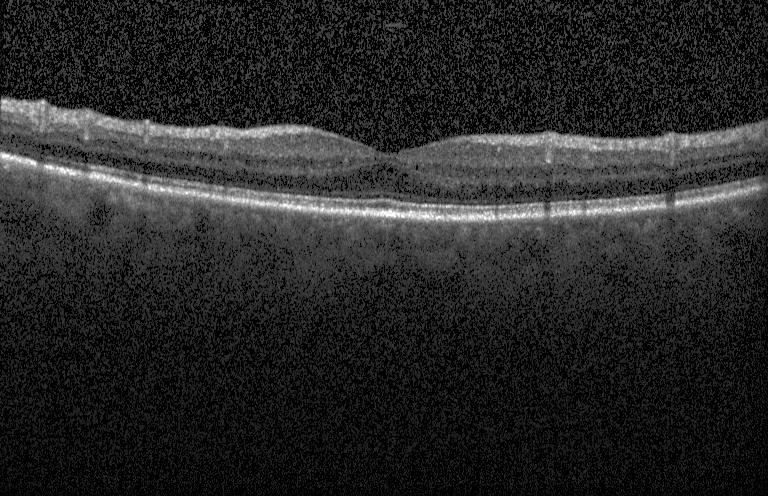

Retinal OCT B-scan — No evidence of CNV, DME, or drusen.